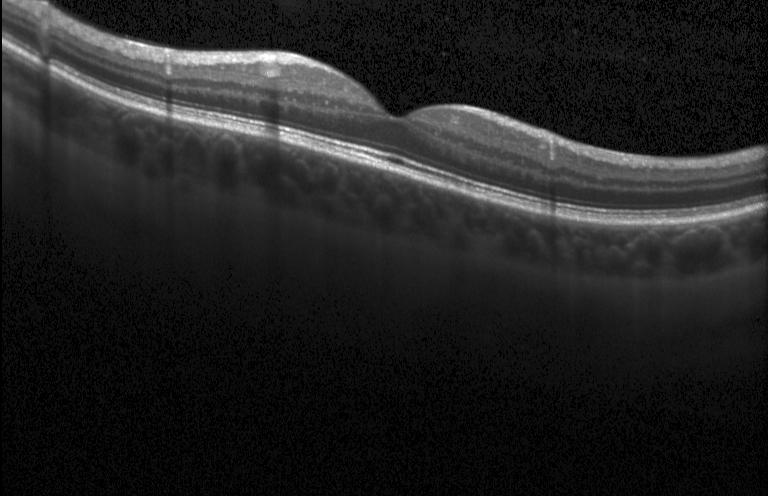 The scan shows no choroidal neovascularization, diabetic macular edema, or drusen.